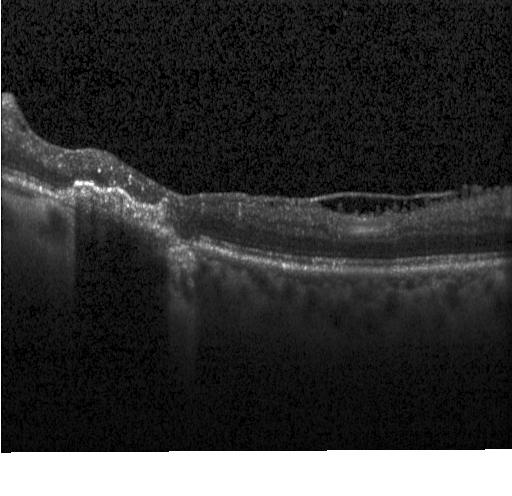 OCT finding: choroidal neovascularization (CNV).